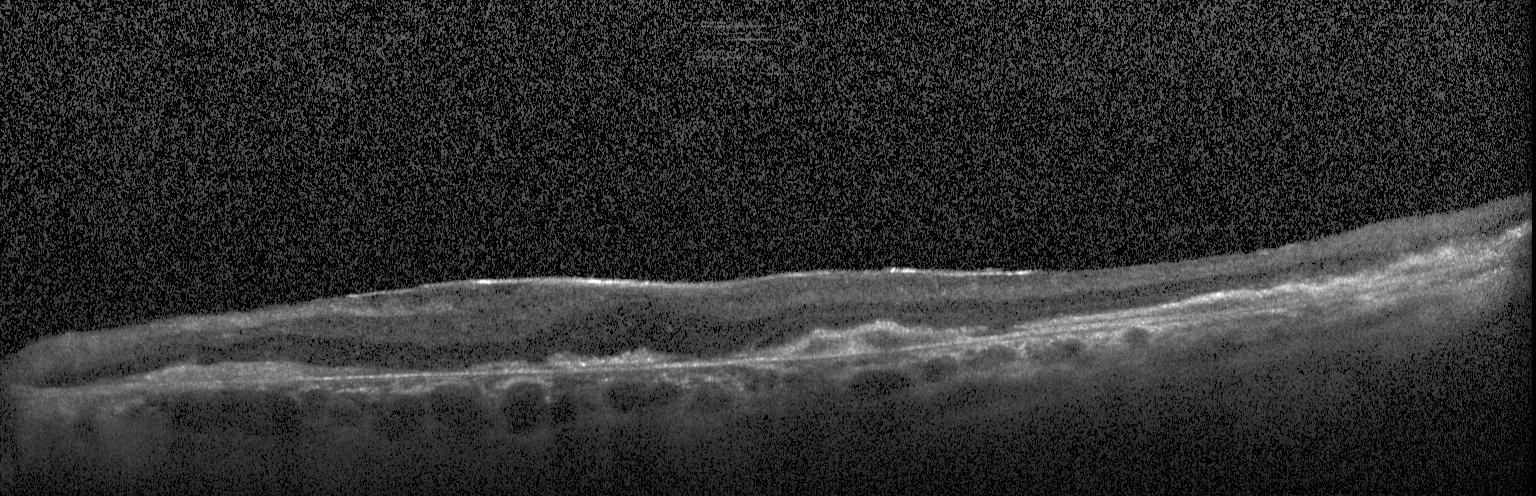

Optical coherence tomography B-scan, acquired on a Heidelberg Spectralis, spectral-domain OCT — Impression: choroidal neovascularization.